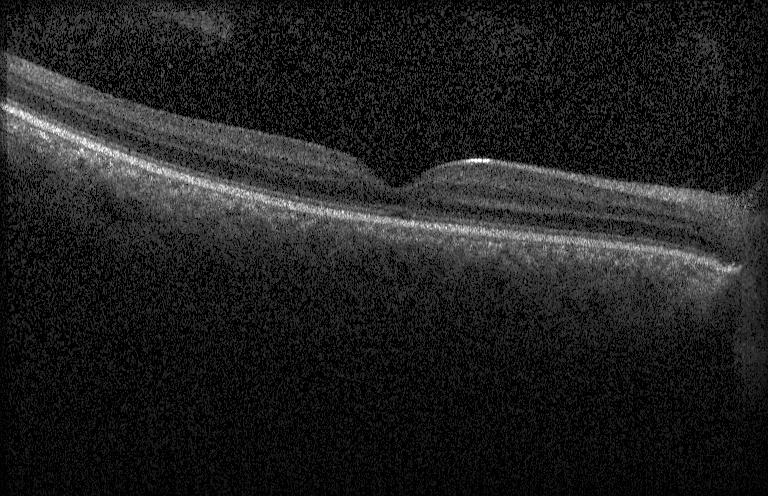

OCT line scan · fovea-centered.
Impression: no CNV, no DME, and no drusen.